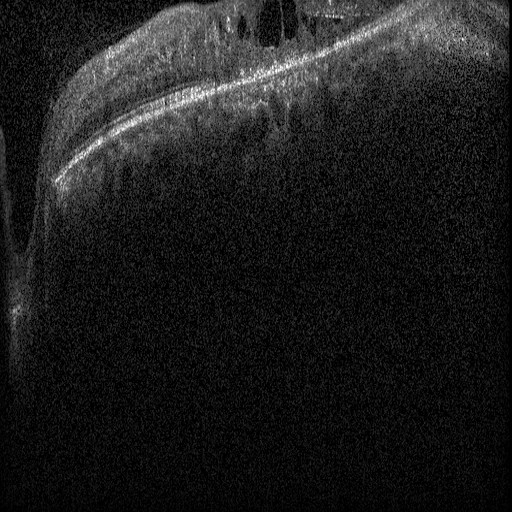 Instrument: Heidelberg Spectralis; macular scan; retinal OCT cross-section; SD-OCT — Assessment: diabetic macular edema (DME).